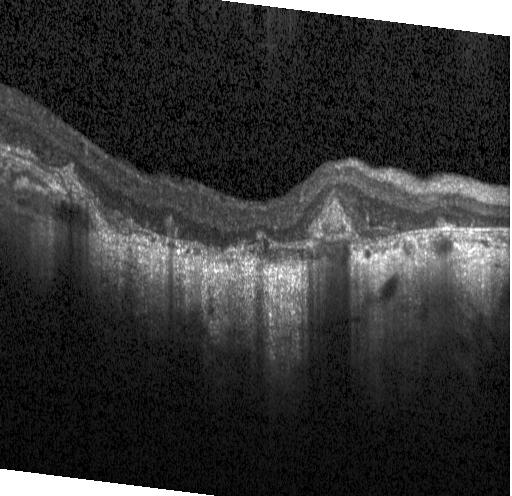

Heidelberg Spectralis OCT system; optical coherence tomography scan; centered on the fovea.
Diagnosis: choroidal neovascularization (CNV).